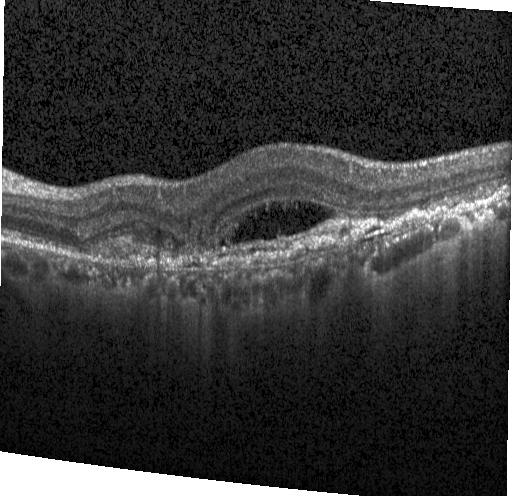 OCT B-scan.
Macular OCT: CNV.